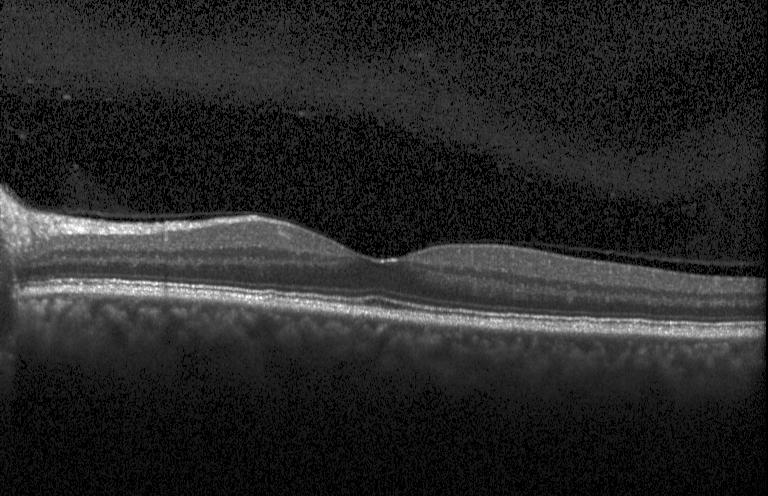

Retinal OCT cross-section. Heidelberg Spectralis OCT system. Dx: no evidence of CNV, DME, or drusen.